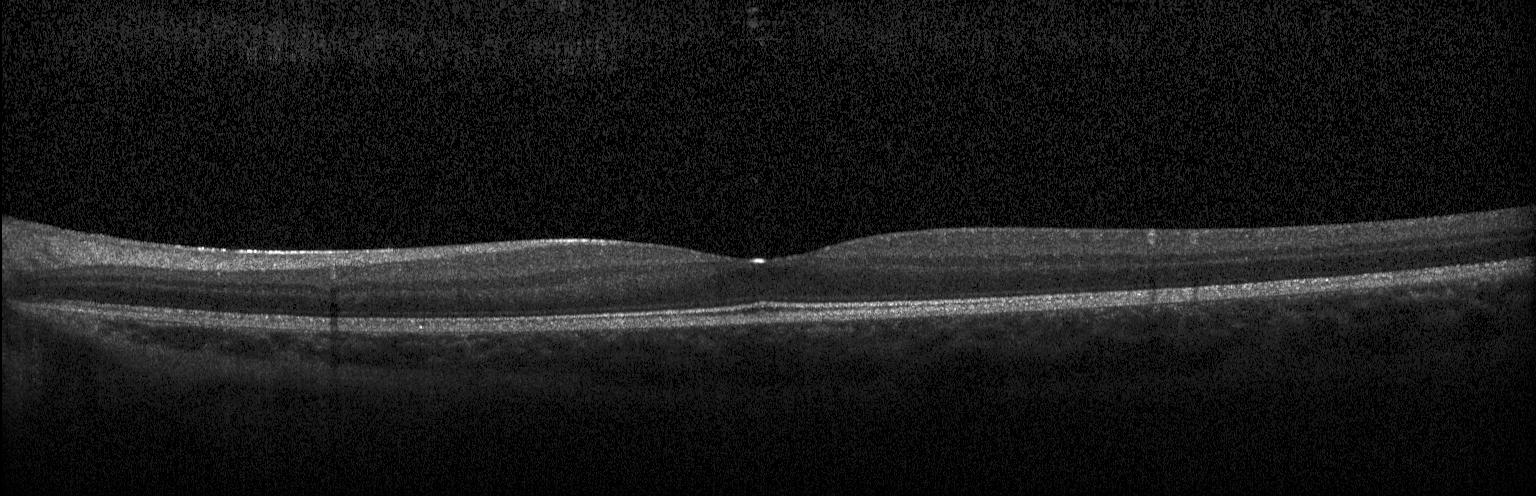 Spectral-domain OCT B-scan: no evidence of CNV, DME, or drusen.